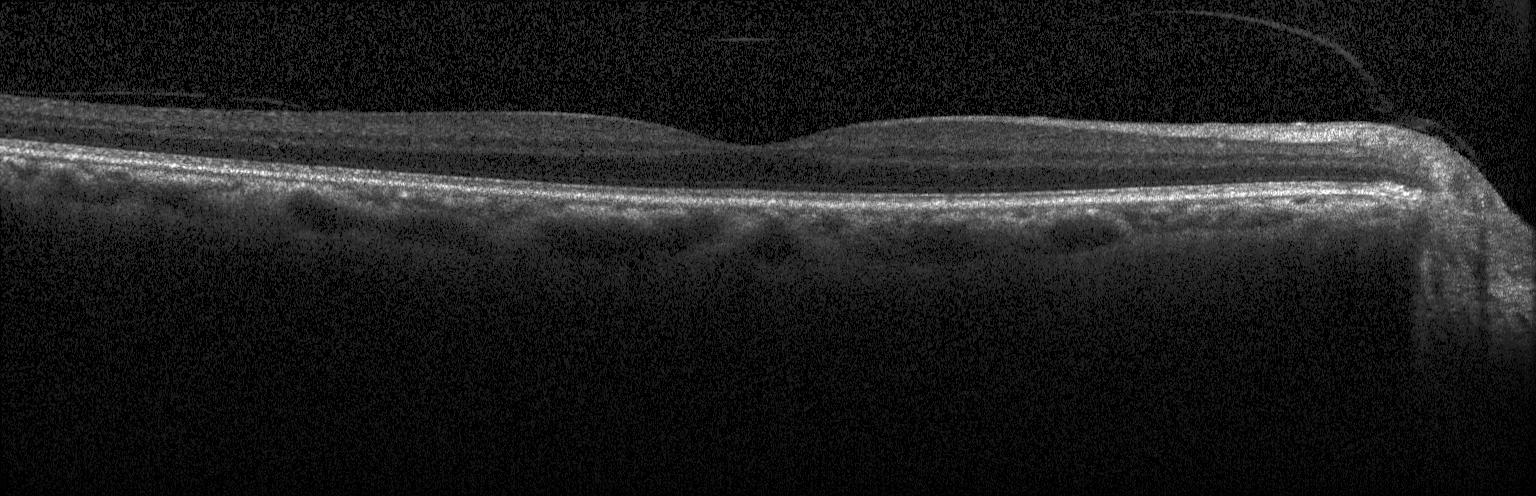

Retinal OCT B-scan — Impression: no evidence of choroidal neovascularization, diabetic macular edema, or drusen.